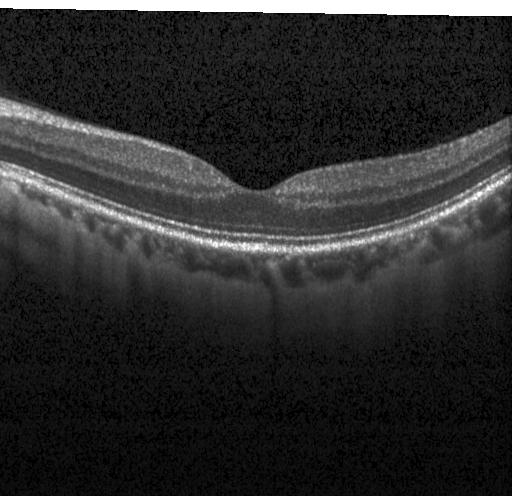

Dx: no evidence of choroidal neovascularization, diabetic macular edema, or drusen.